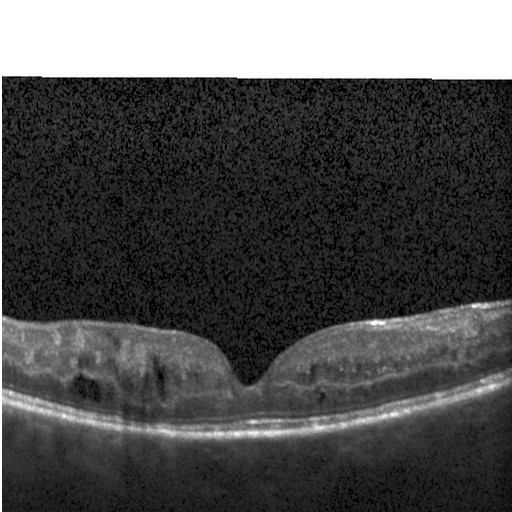 Retinal OCT cross-section. Finding: diabetic macular edema.